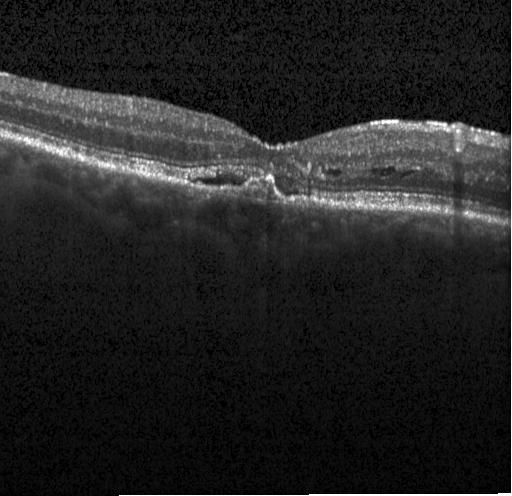
Fovea-centered · instrument: Heidelberg Spectralis · OCT B-scan — Macular OCT: a choroidal neovascular membrane.